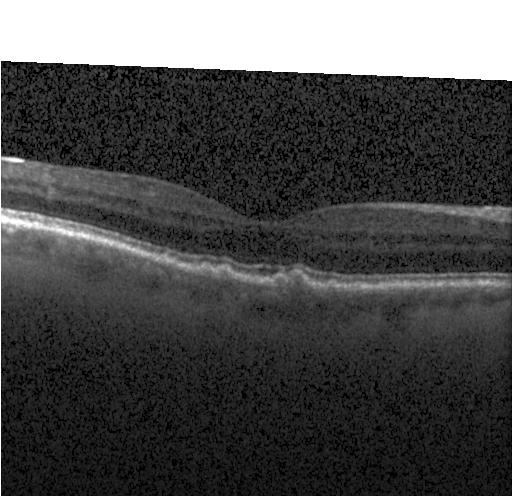
Retinal OCT B-scan, fovea-centered.
The scan shows multiple drusen.